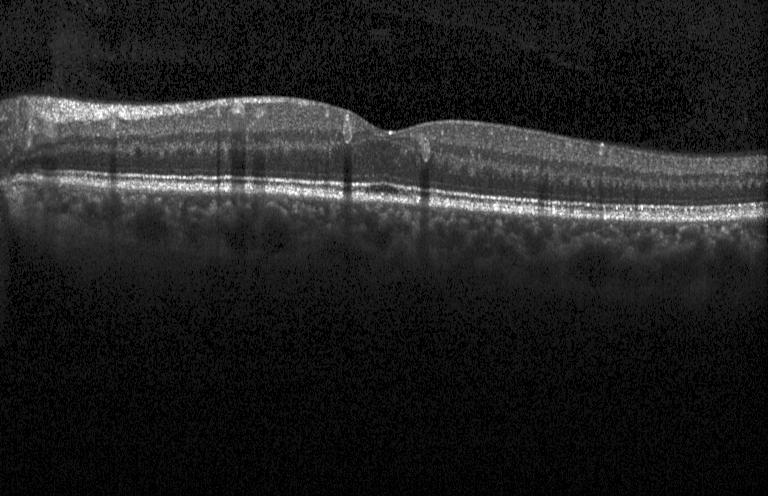
Impression: no choroidal neovascularization, no diabetic macular edema, and no drusen.